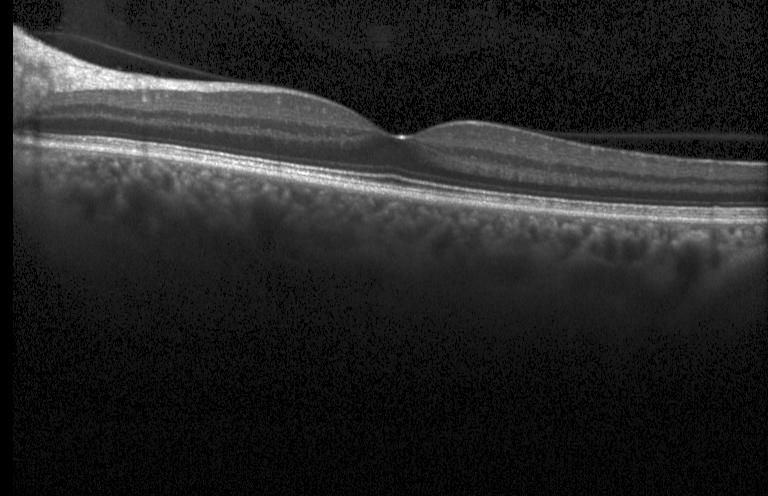
Retinal OCT cross-section showing no choroidal neovascularization, diabetic macular edema, or drusen.